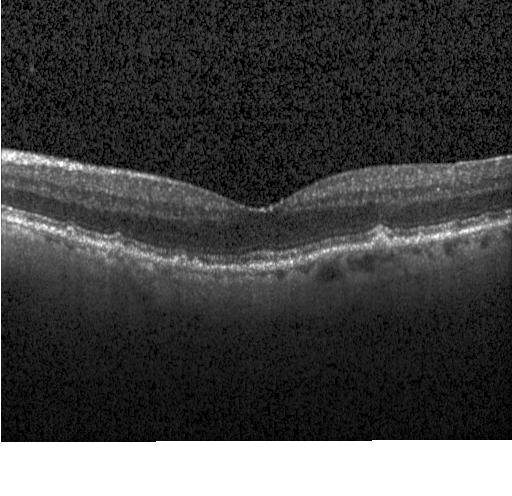

Optical coherence tomography B-scan; instrument: Heidelberg Spectralis; macular scan.
Diagnosis: sub-RPE drusenoid deposits.